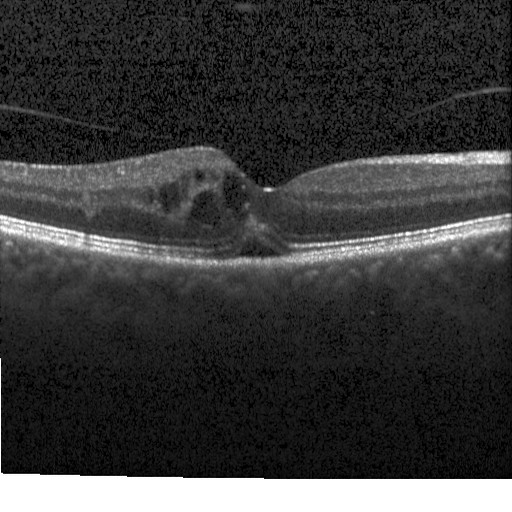 Instrument: Heidelberg Spectralis; spectral-domain OCT; optical coherence tomography B-scan.
This B-scan demonstrates diabetic macular edema (DME).